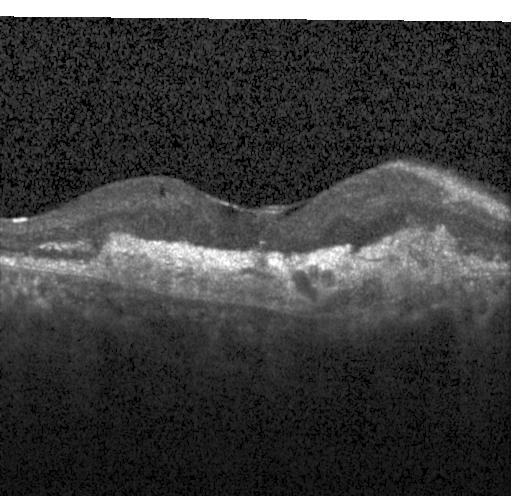

The scan shows choroidal neovascularization (CNV).